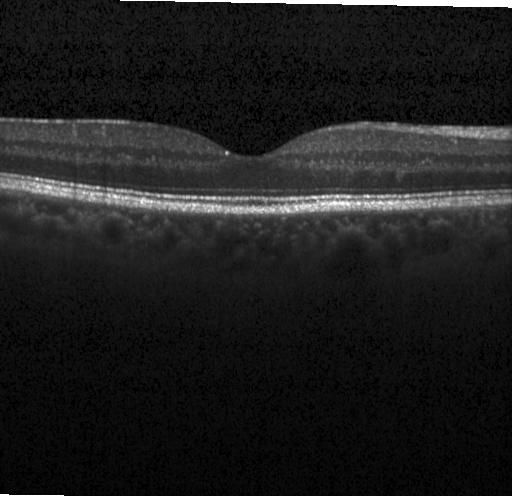

Diagnosis: no evidence of choroidal neovascularization, diabetic macular edema, or drusen.